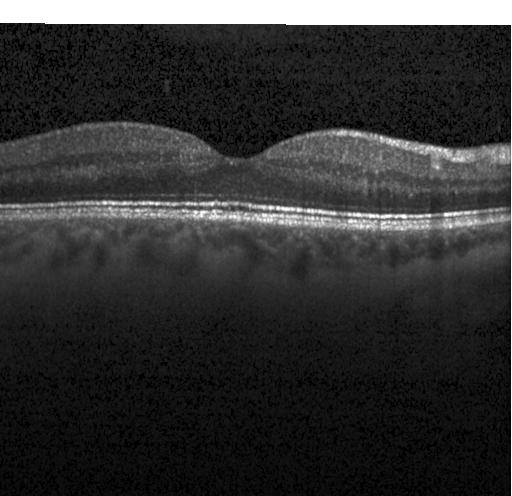

Optical coherence tomography scan; macular scan; acquired on a Heidelberg Spectralis; spectral-domain OCT — Dx: no evidence of choroidal neovascularization, diabetic macular edema, or drusen.